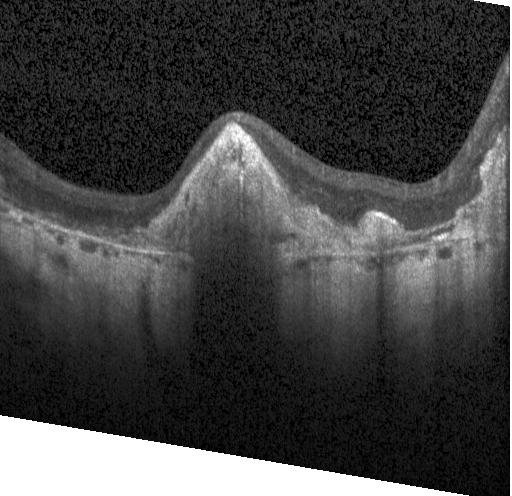
Finding: choroidal neovascularization.